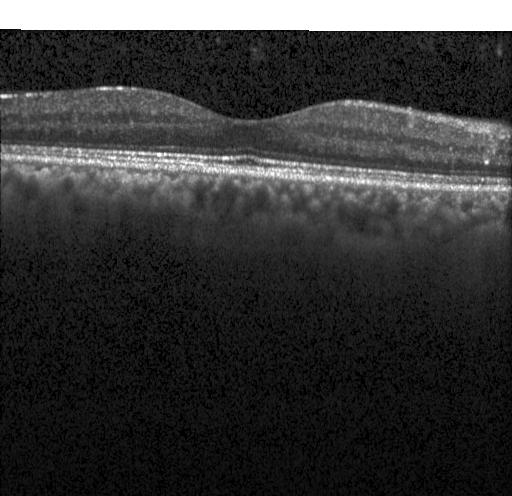

OCT B-scan
Neither choroidal neovascularization, diabetic macular edema, nor drusen.